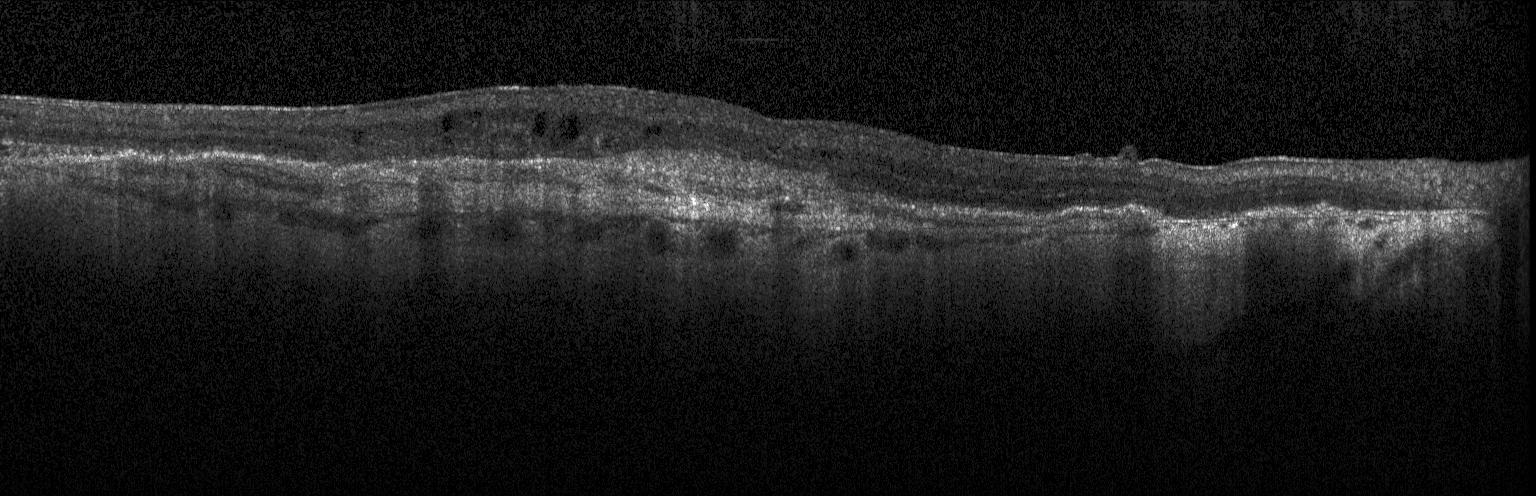 Dx: choroidal neovascularization.